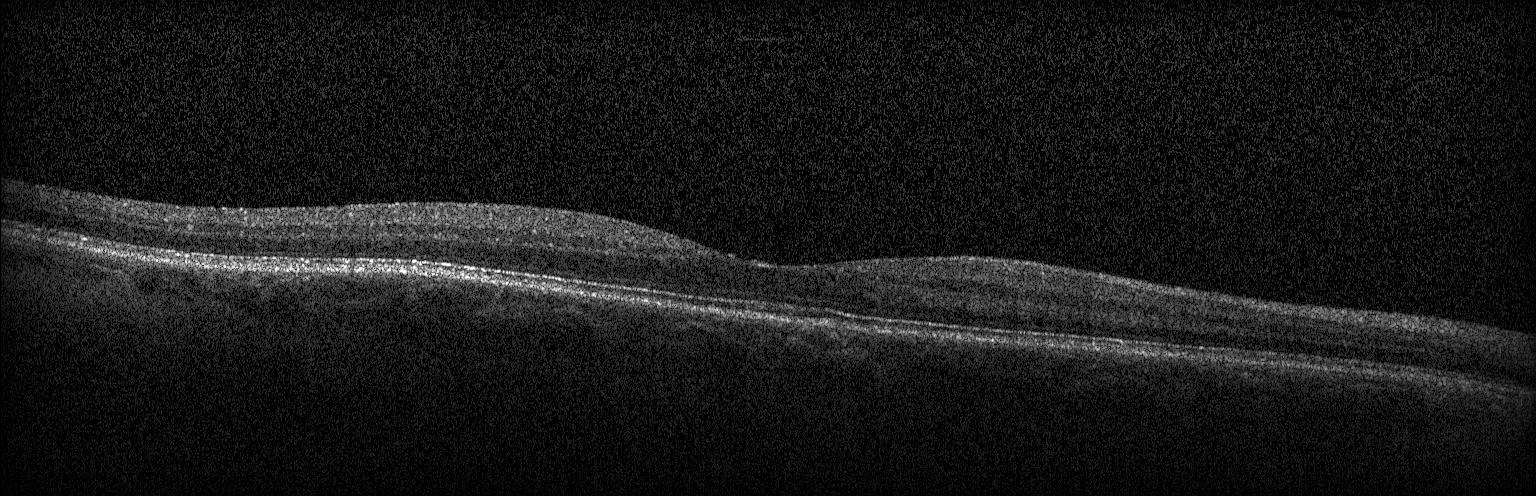

Diagnosis: no choroidal neovascularization, diabetic macular edema, or drusen.